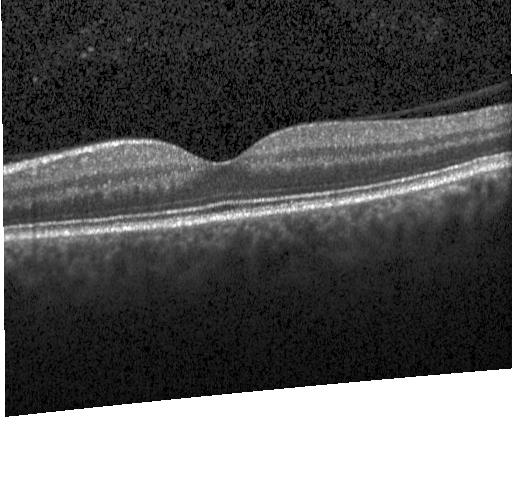 Macular OCT: neither CNV, DME, nor drusen.